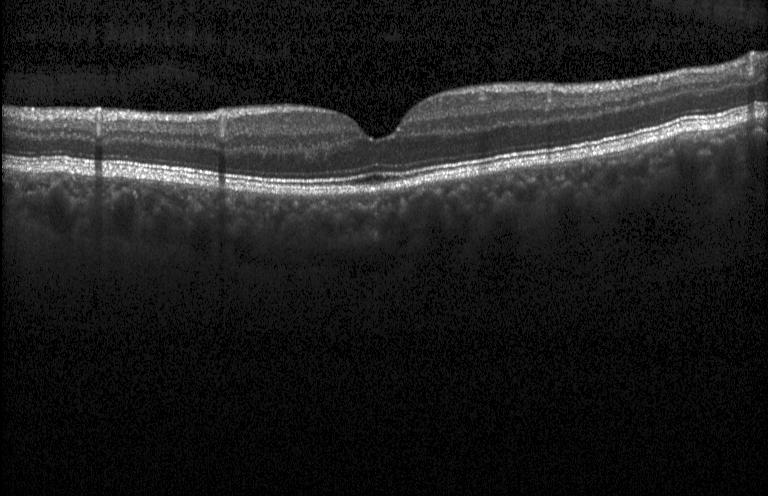 Optical coherence tomography scan
Impression: no CNV, no DME, and no drusen.